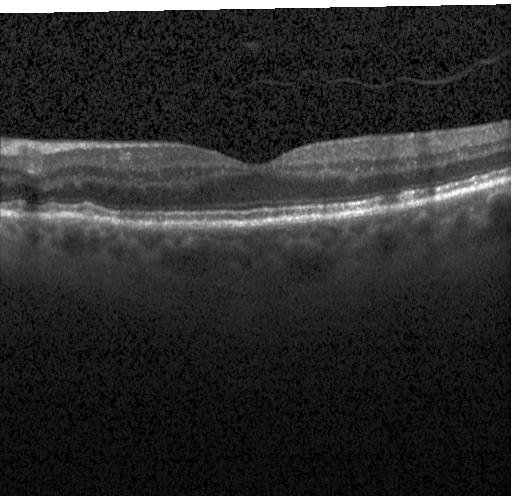

Optical coherence tomography scan; spectral-domain optical coherence tomography; Heidelberg Spectralis OCT system. OCT finding: drusen.